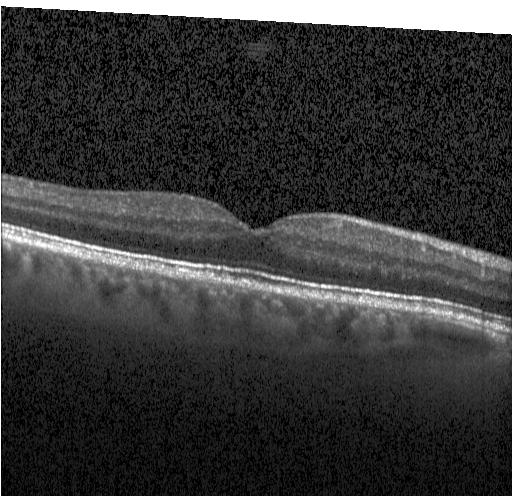
Retinal OCT B-scan · acquired on a Heidelberg Spectralis.
No choroidal neovascularization, diabetic macular edema, or drusen.